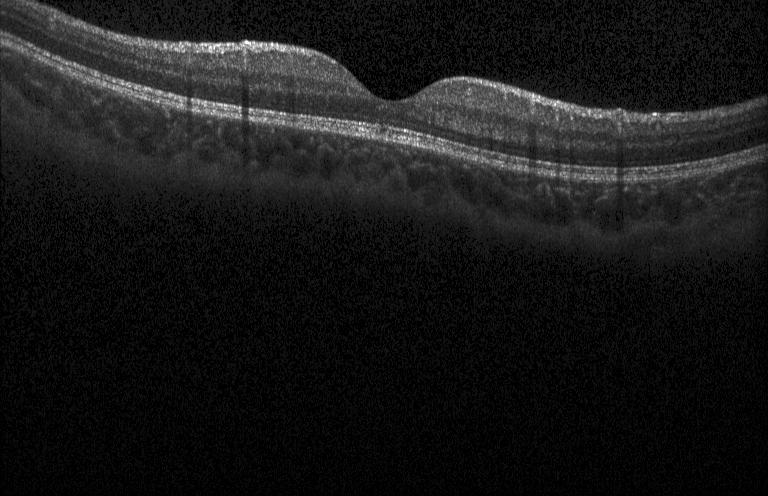
Finding: neither CNV, DME, nor drusen.